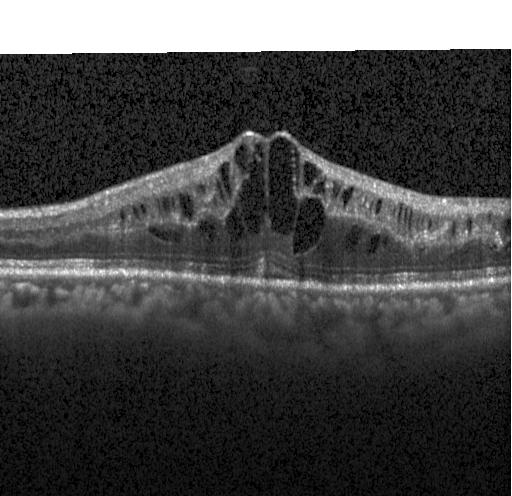

Optical coherence tomography B-scan. Finding: diabetic macular edema (DME).